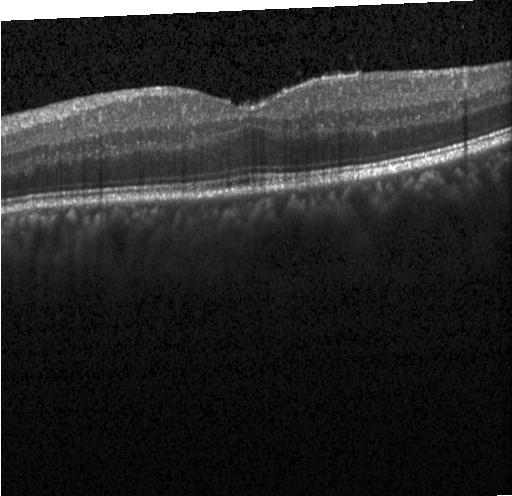
Retinal OCT B-scan · SD-OCT · Heidelberg Spectralis OCT system · macular scan
Diagnosis: neither choroidal neovascularization, diabetic macular edema, nor drusen.